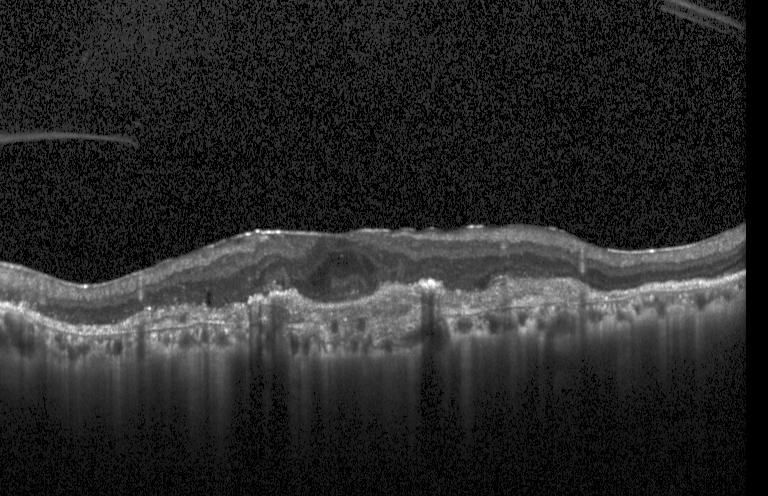
Heidelberg Spectralis OCT system; horizontal scan through the fovea; retinal OCT cross-section. Dx: a choroidal neovascular membrane.